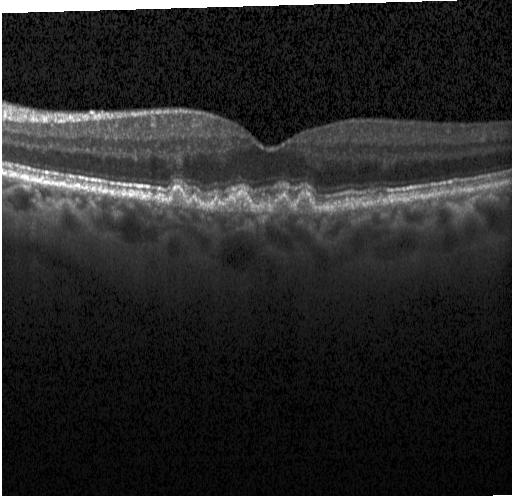 Macular OCT demonstrating sub-RPE drusenoid deposits.